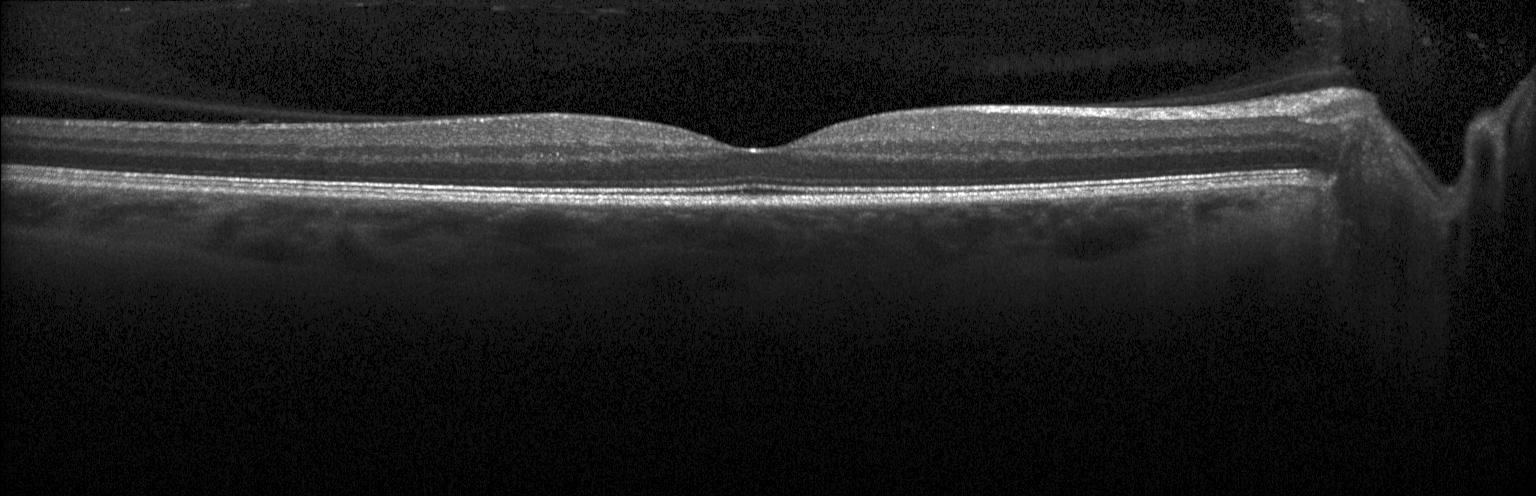 Dx: no evidence of choroidal neovascularization, diabetic macular edema, or drusen.